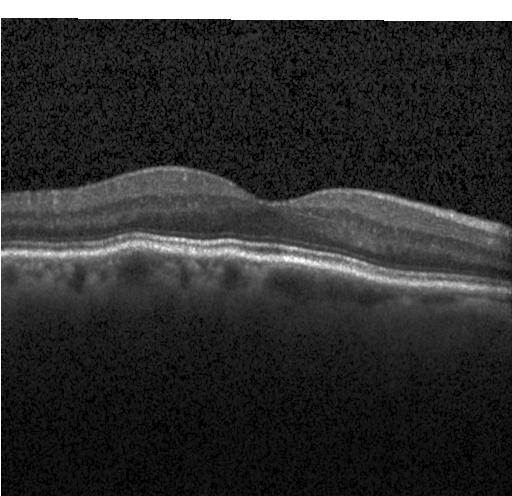 Assessment: no CNV, no DME, and no drusen.